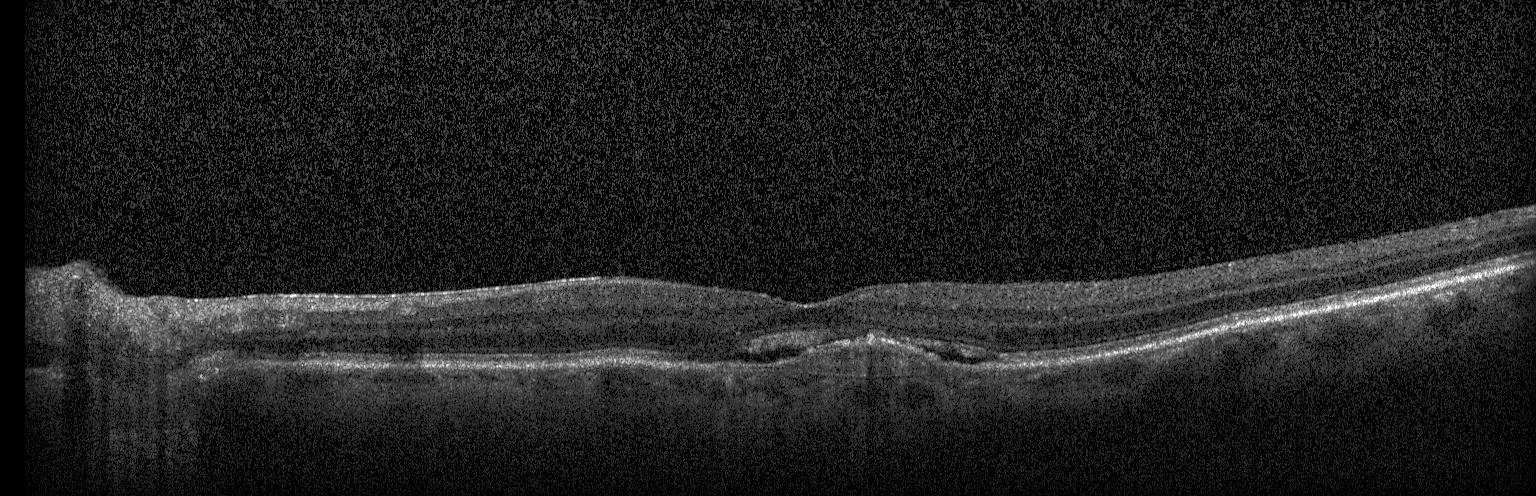

Horizontal scan through the fovea; OCT B-scan.
Assessment: choroidal neovascularization.